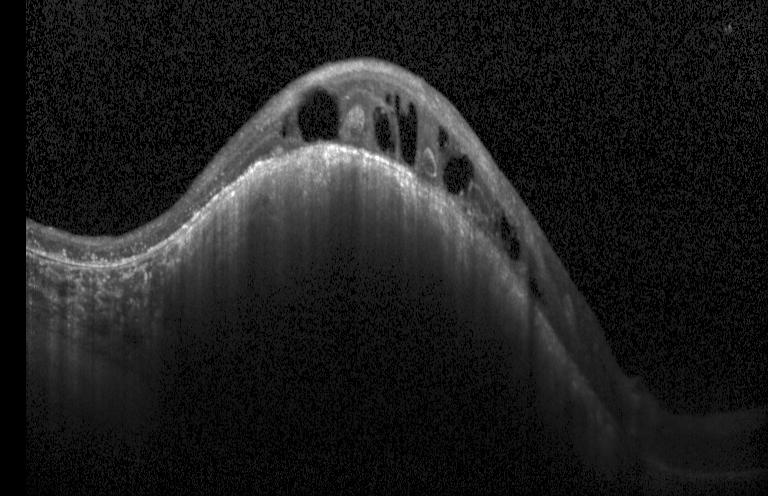

The scan shows DME.